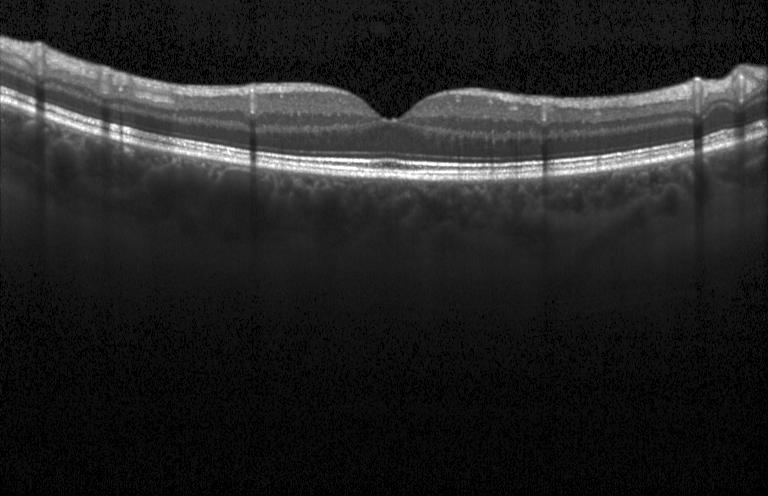
Macular OCT demonstrating neither CNV, DME, nor drusen.